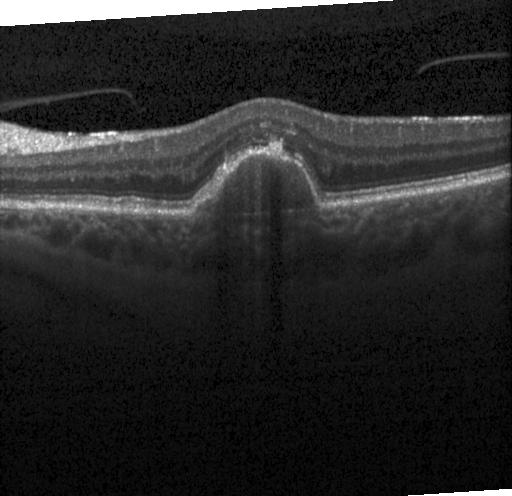
Finding: CNV.